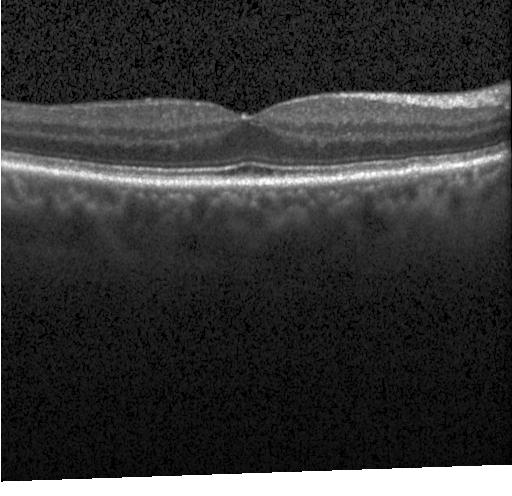 OCT finding: no choroidal neovascularization, diabetic macular edema, or drusen.